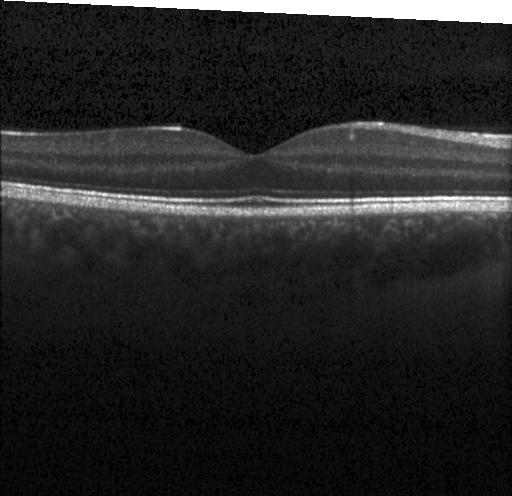 Spectral-domain OCT B-scan: no choroidal neovascularization, no diabetic macular edema, and no drusen.